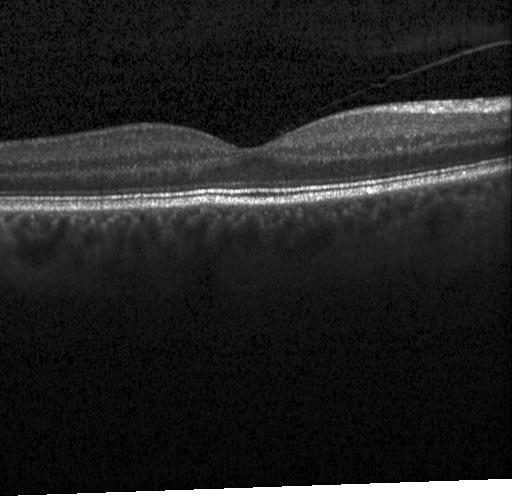 Optical coherence tomography scan
Finding: no choroidal neovascularization, diabetic macular edema, or drusen.